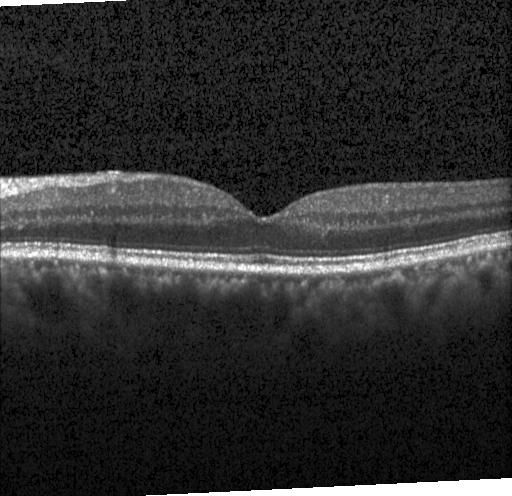 Fovea-centered, spectral-domain optical coherence tomography, optical coherence tomography scan.
Diagnosis: no evidence of CNV, DME, or drusen.